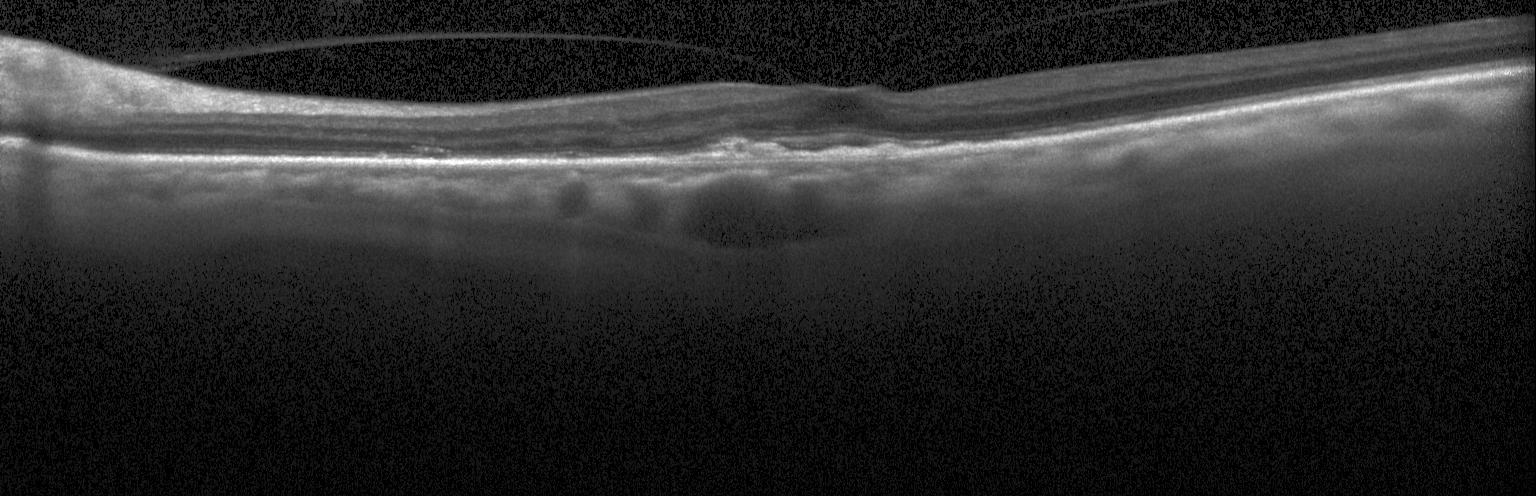

Impression: a choroidal neovascular membrane.